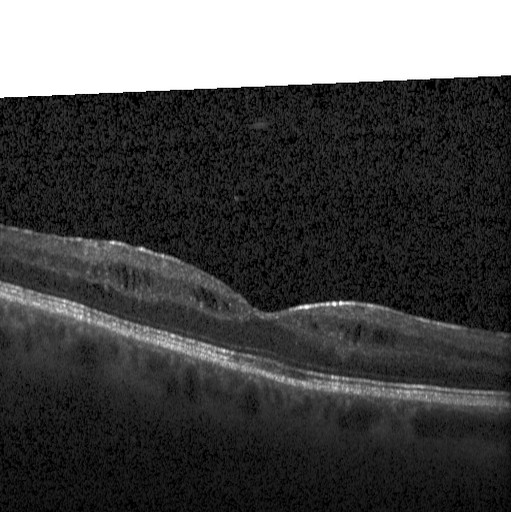
Horizontal scan through the fovea · retinal OCT cross-section · acquired on a Heidelberg Spectralis · spectral-domain optical coherence tomography.
OCT finding: diabetic macular edema (DME).